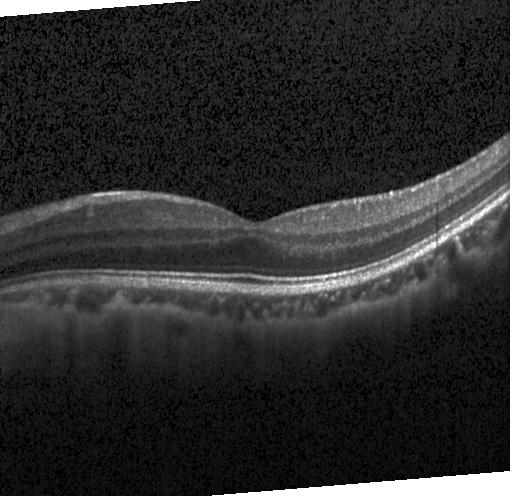 Centered on the fovea. Retinal OCT B-scan. Heidelberg Spectralis OCT system. Macular OCT: no evidence of CNV, DME, or drusen.